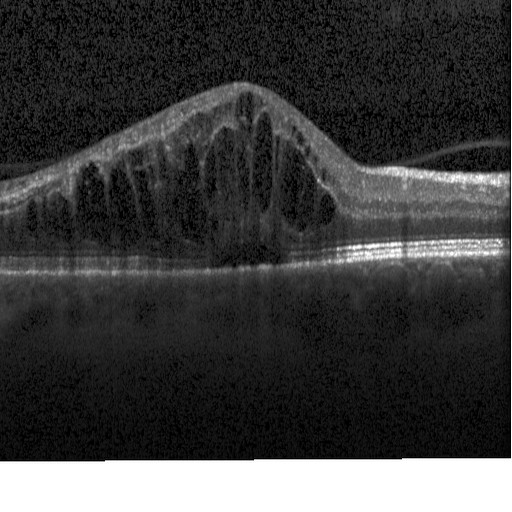
The scan shows DME.